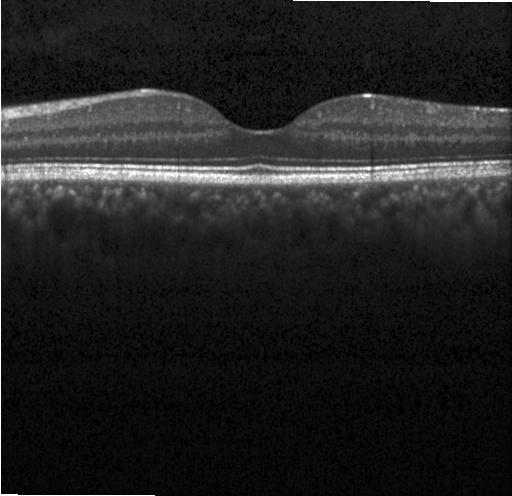
Through the macula · Heidelberg Spectralis OCT system · optical coherence tomography scan
No CNV, DME, or drusen.